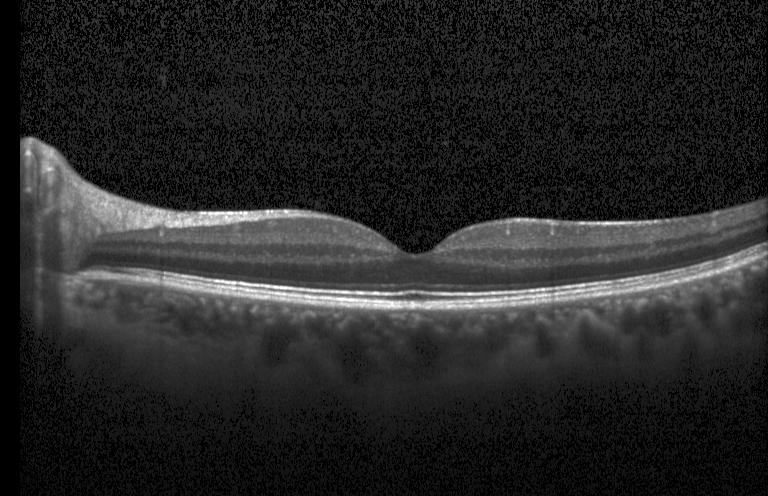 Retinal OCT cross-section.
Impression: no choroidal neovascularization, no diabetic macular edema, and no drusen.